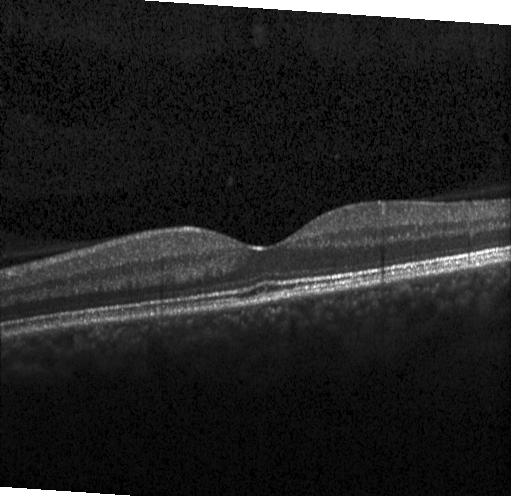

Retinal OCT cross-section, fovea-centered, spectral-domain OCT, acquired on a Heidelberg Spectralis.
Assessment: neither choroidal neovascularization, diabetic macular edema, nor drusen.